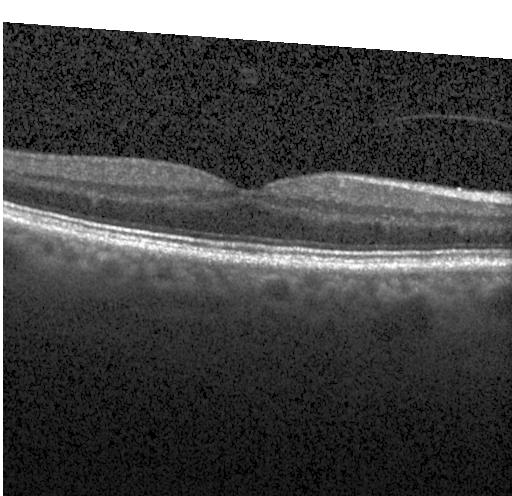
OCT B-scan · through the macula.
Diagnosis: neither choroidal neovascularization, diabetic macular edema, nor drusen.